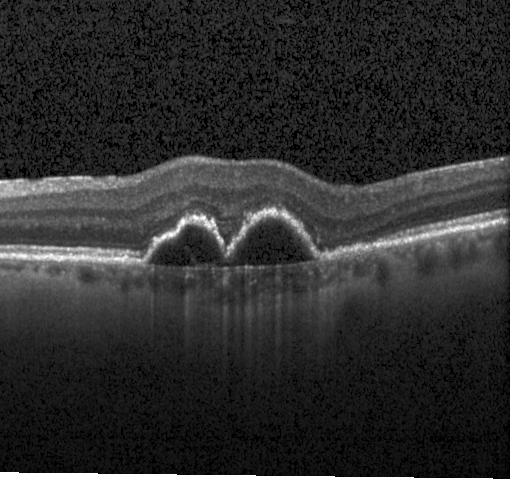

Optical coherence tomography B-scan · through the macula. This B-scan demonstrates choroidal neovascularization.